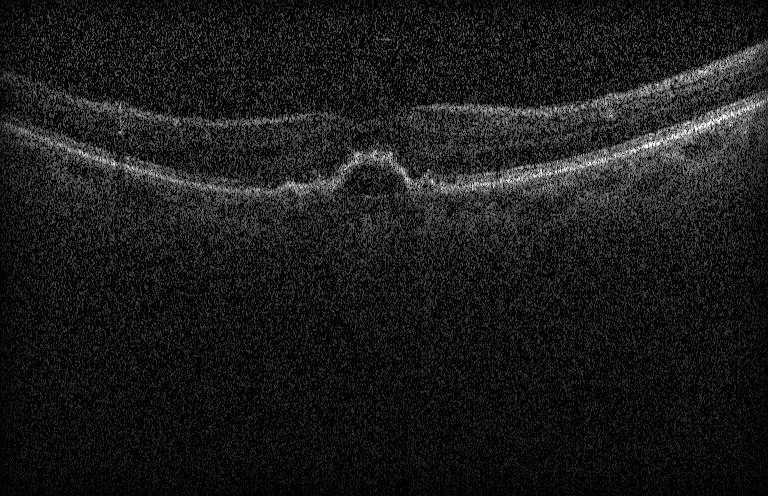
OCT line scan.
Impression: choroidal neovascularization (CNV).